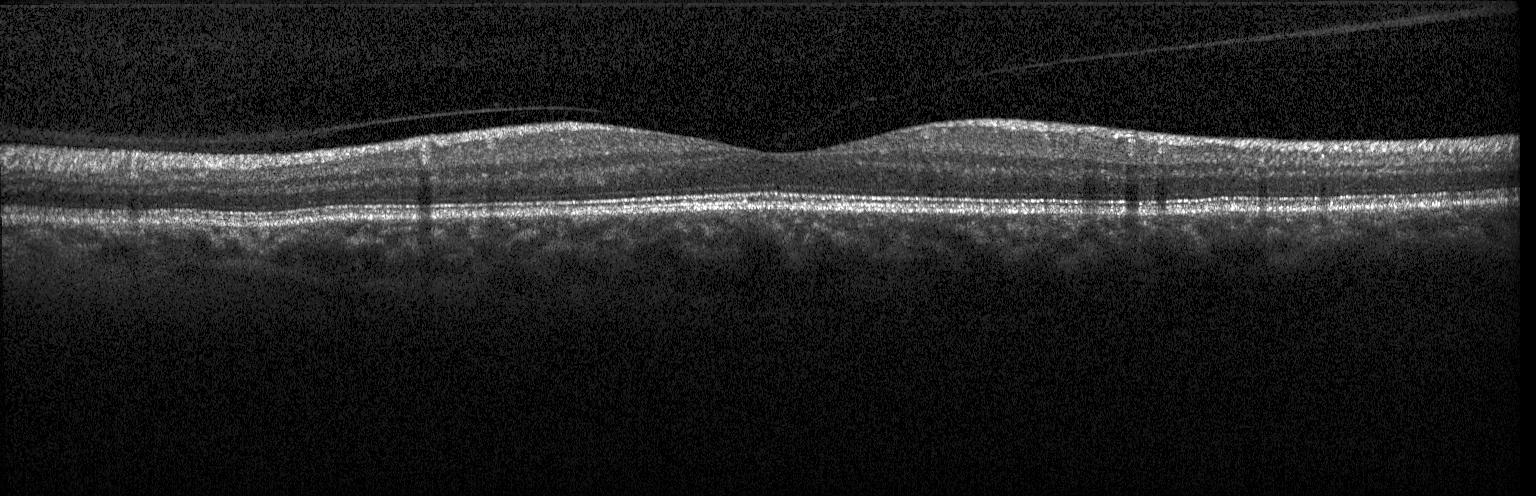

Optical coherence tomography scan · spectral-domain OCT · acquired on a Heidelberg Spectralis · horizontal scan through the fovea — Finding: neither choroidal neovascularization, diabetic macular edema, nor drusen.